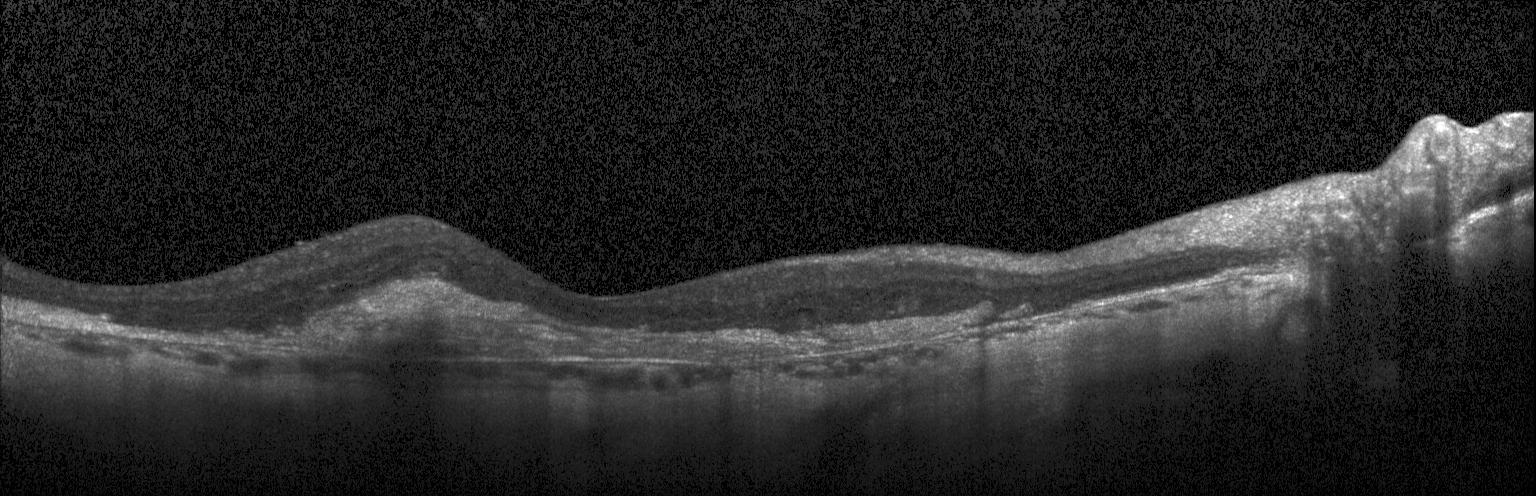

Instrument: Heidelberg Spectralis. Macular scan. Retinal OCT cross-section
Diagnosis: a choroidal neovascular membrane.